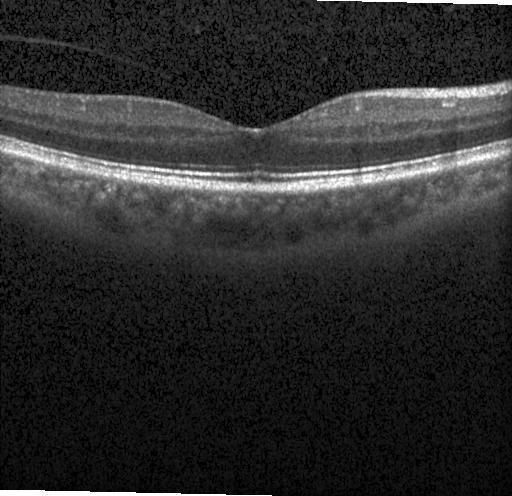 OCT B-scan showing no CNV, no DME, and no drusen.